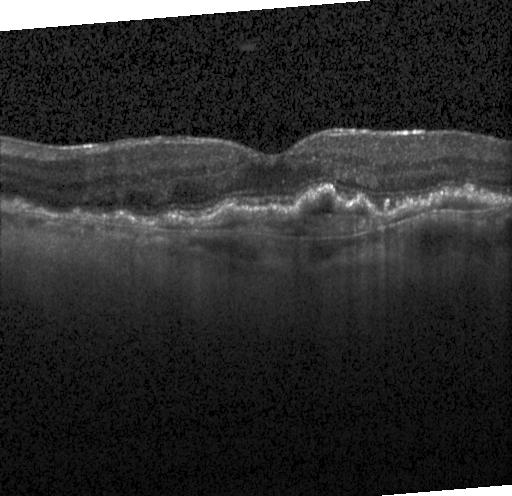

Spectral-domain optical coherence tomography; optical coherence tomography scan.
Finding: a choroidal neovascular membrane.